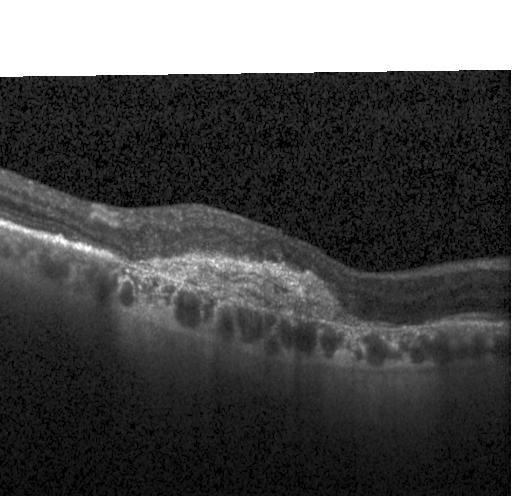
SD-OCT · acquired on a Heidelberg Spectralis · OCT B-scan. Diagnosis: a choroidal neovascular membrane.